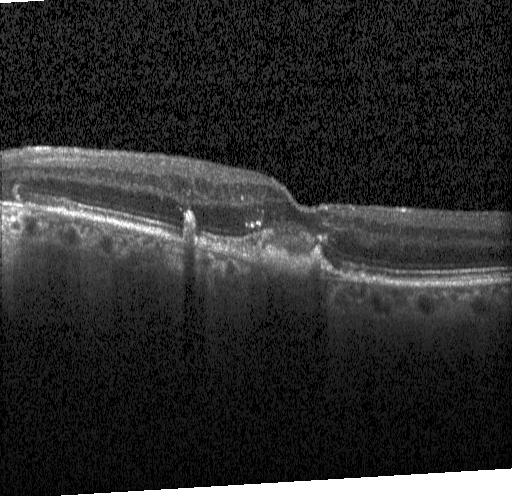 OCT B-scan. Horizontal scan through the fovea.
Finding: a choroidal neovascular membrane.